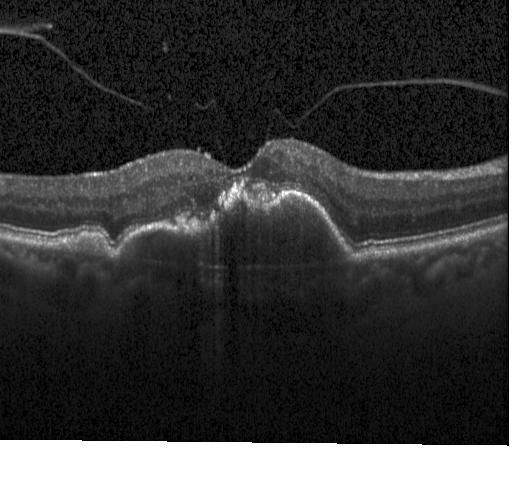

Through the macula · OCT line scan · Heidelberg Spectralis — A choroidal neovascular membrane.